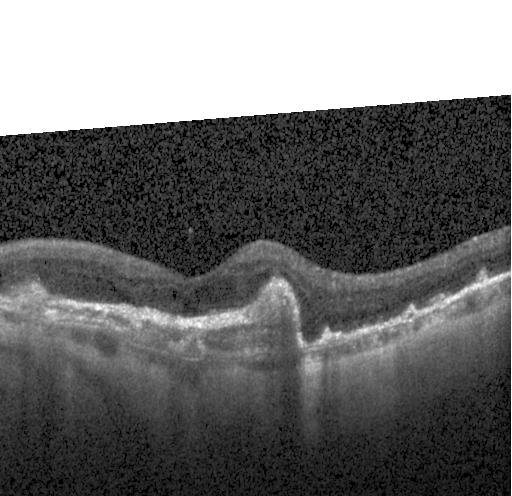

Retinal OCT cross-section showing a choroidal neovascular membrane.